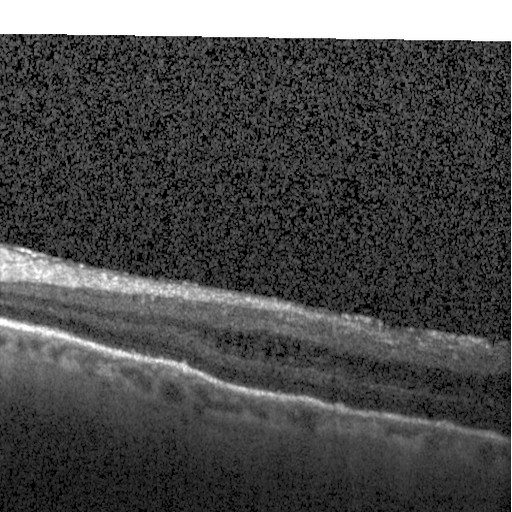 Acquired on a Heidelberg Spectralis; spectral-domain OCT; fovea-centered; optical coherence tomography scan — Diagnosis: diabetic macular edema (DME).